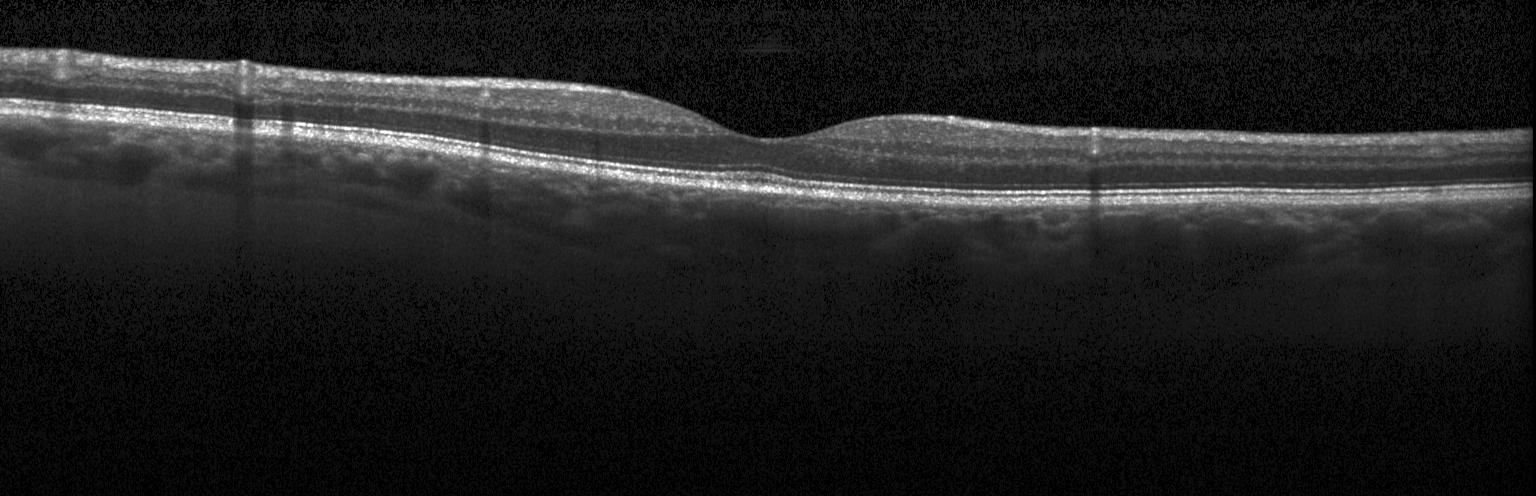
Centered on the fovea · OCT B-scan
Diagnosis: no choroidal neovascularization, diabetic macular edema, or drusen.